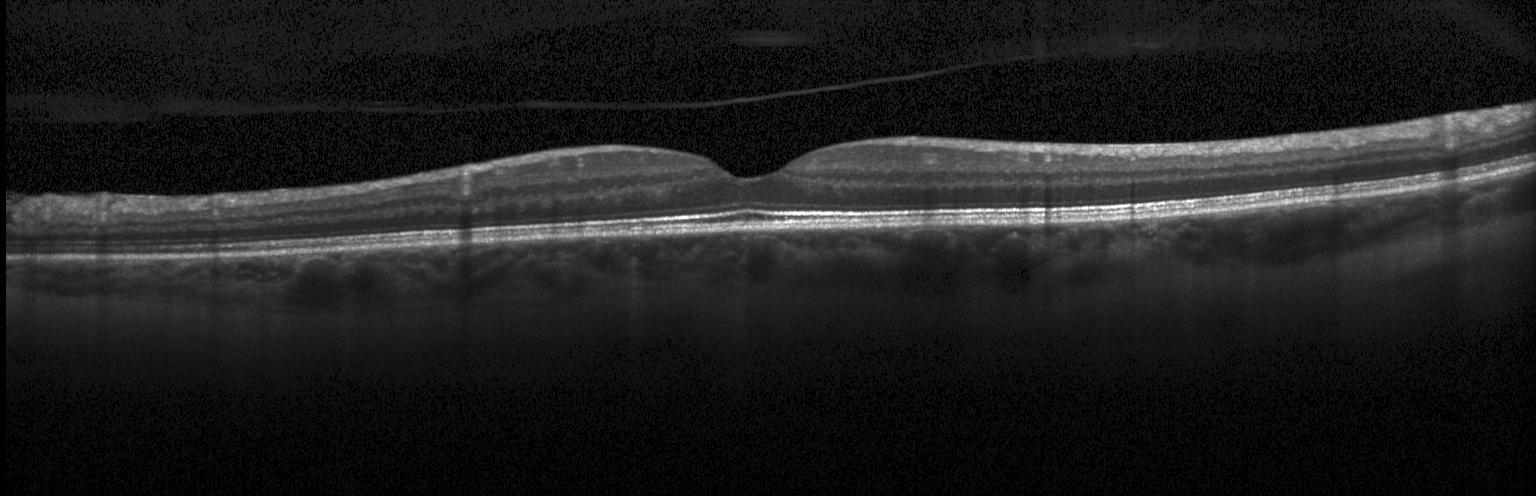

Finding: no choroidal neovascularization, diabetic macular edema, or drusen.